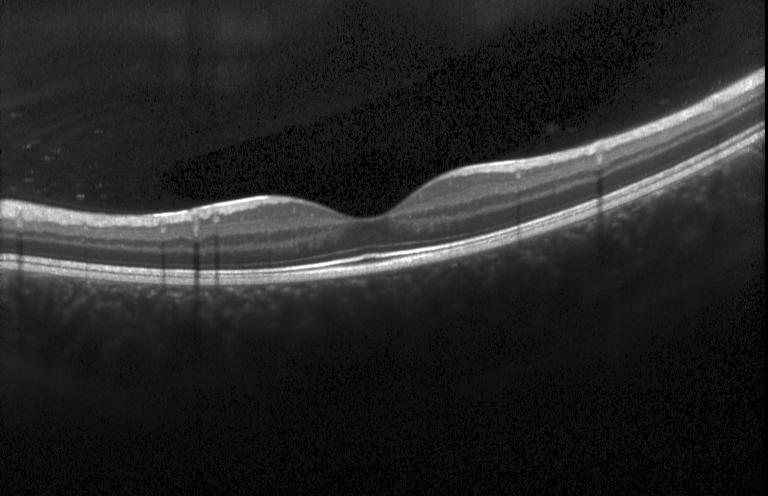
Centered on the fovea · acquired on a Heidelberg Spectralis · retinal OCT B-scan · SD-OCT. Finding: no choroidal neovascularization, no diabetic macular edema, and no drusen.